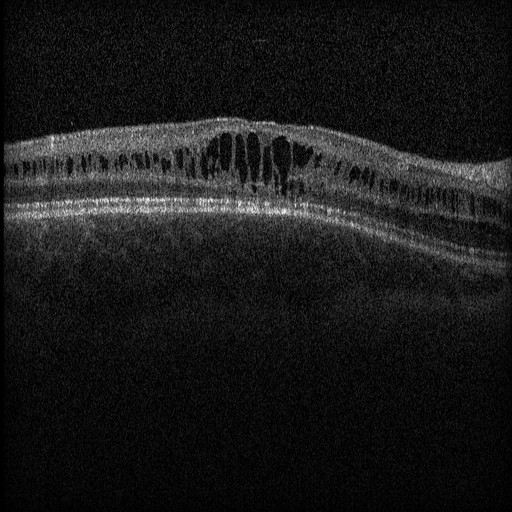 Impression: DME.